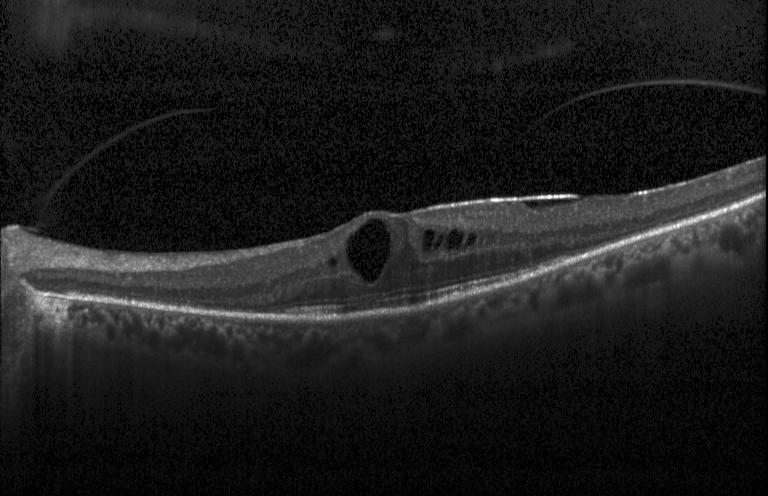

Spectral-domain optical coherence tomography. OCT B-scan. Diagnosis: diabetic macular edema (DME).